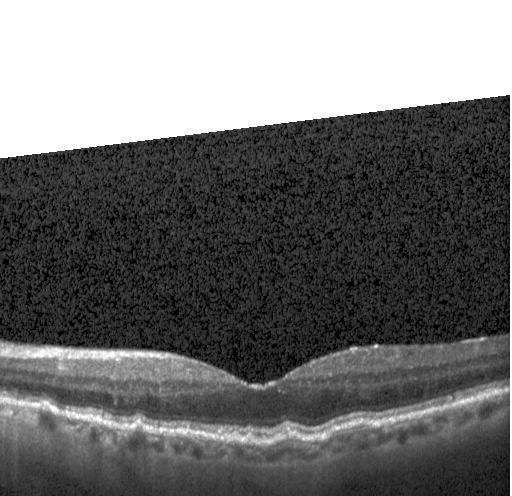

Impression: a choroidal neovascular membrane.